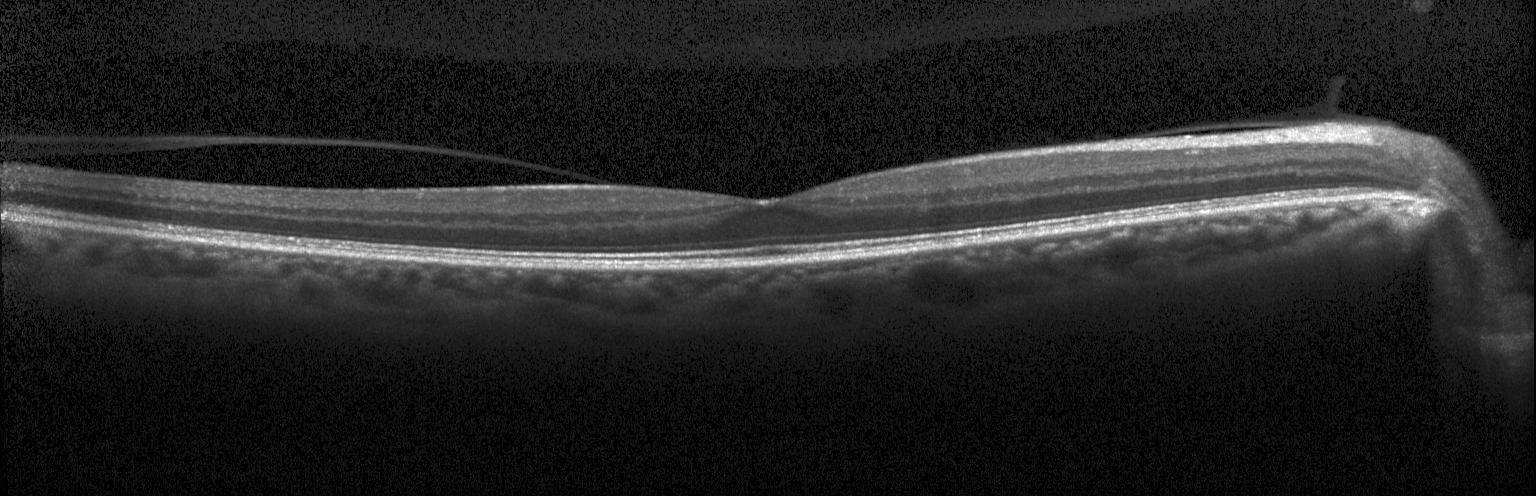

Centered on the fovea · spectral-domain OCT · OCT line scan
Assessment: neither choroidal neovascularization, diabetic macular edema, nor drusen.